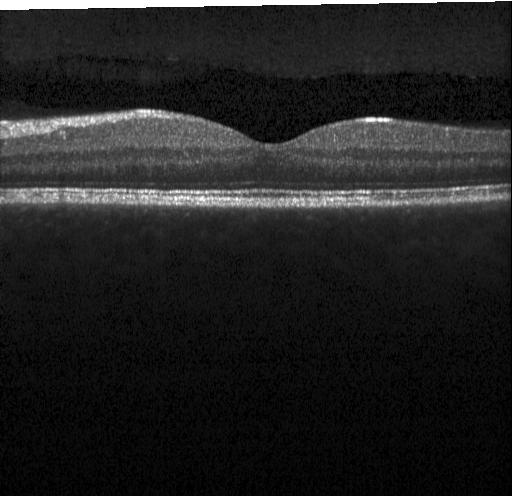

Dx: no evidence of choroidal neovascularization, diabetic macular edema, or drusen.